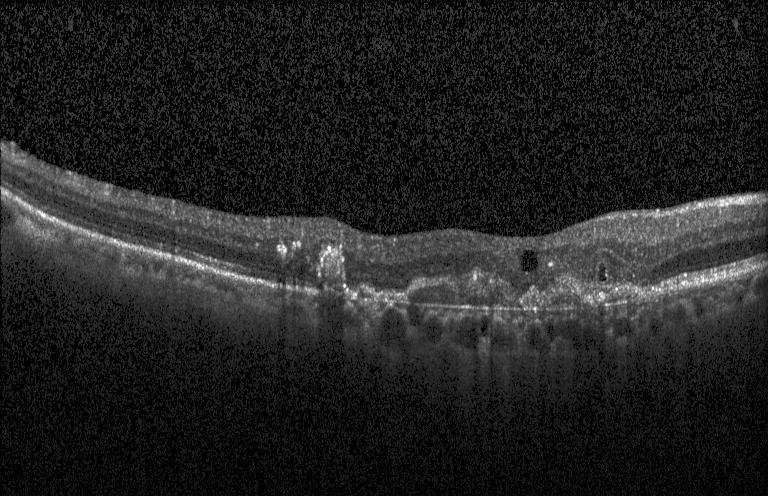

OCT line scan — Diagnosis: choroidal neovascularization (CNV).